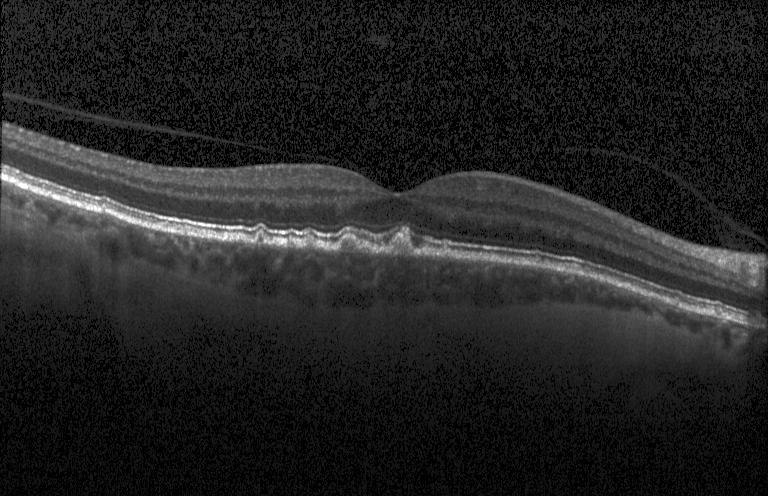 Through the macula · retinal OCT cross-section · acquired on a Heidelberg Spectralis
Macular OCT: drusen.